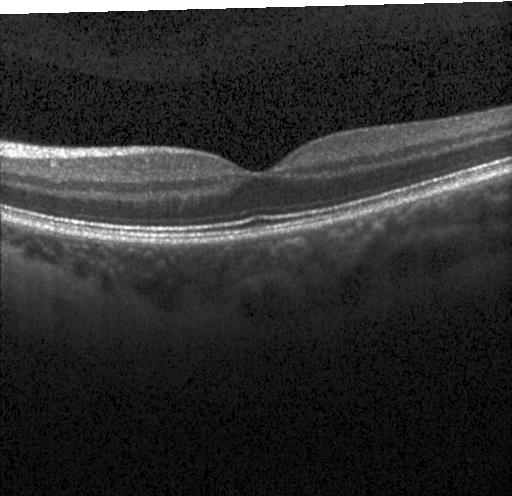
Optical coherence tomography B-scan · horizontal scan through the fovea.
Macular OCT: no choroidal neovascularization, diabetic macular edema, or drusen.